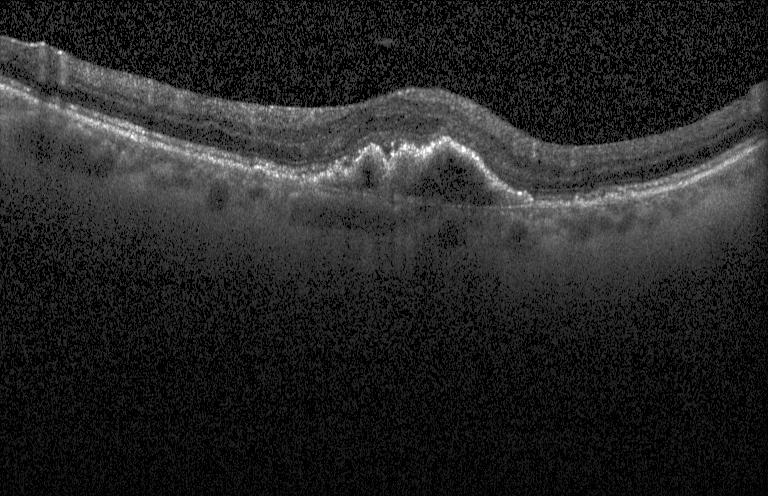

Diagnosis: choroidal neovascularization (CNV).